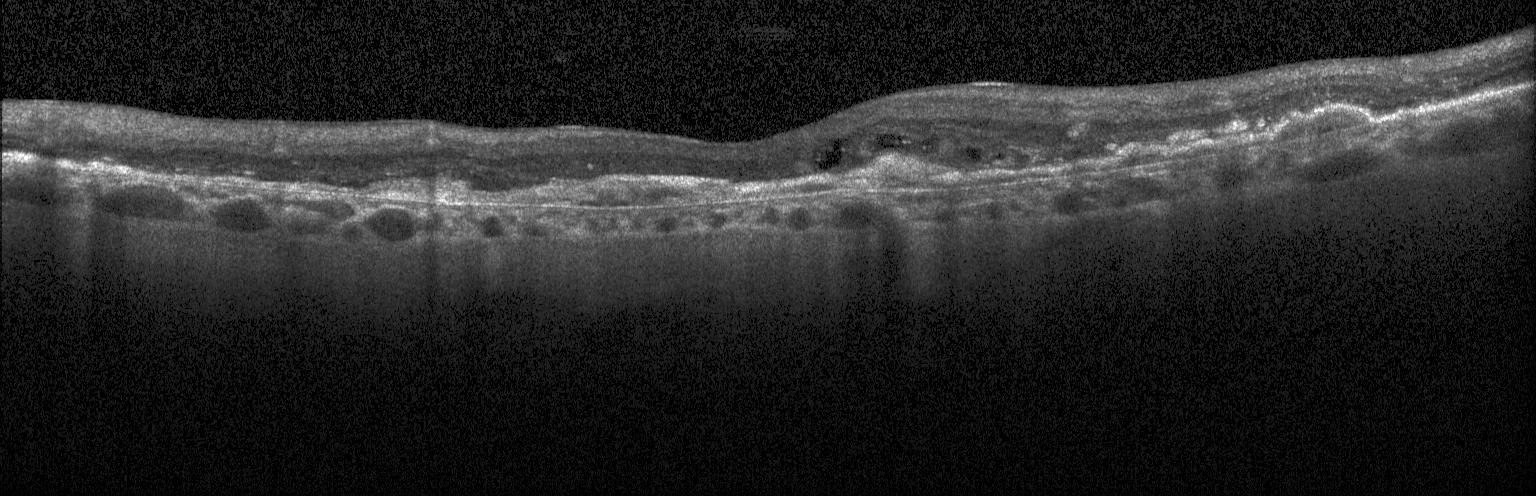

Retinal OCT cross-section. Finding: choroidal neovascularization.